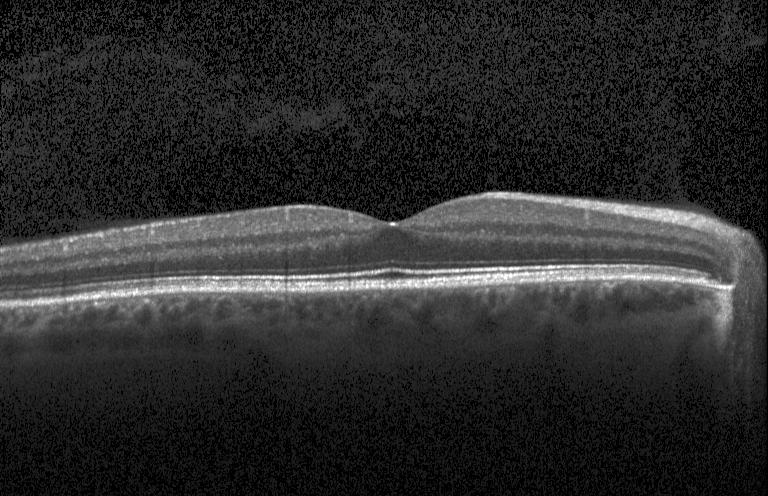
Heidelberg Spectralis OCT system; OCT line scan; through the macula; SD-OCT — Impression: neither choroidal neovascularization, diabetic macular edema, nor drusen.